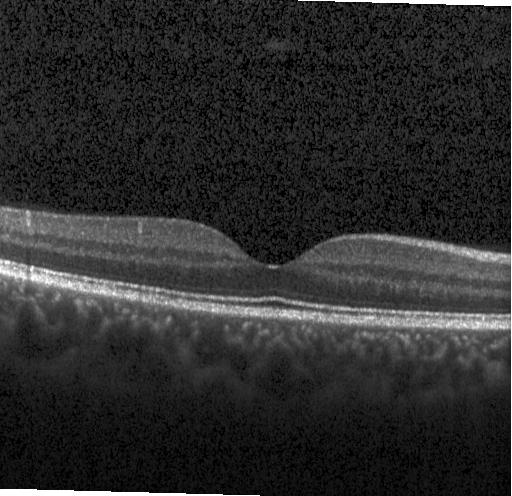

Impression: no evidence of choroidal neovascularization, diabetic macular edema, or drusen.